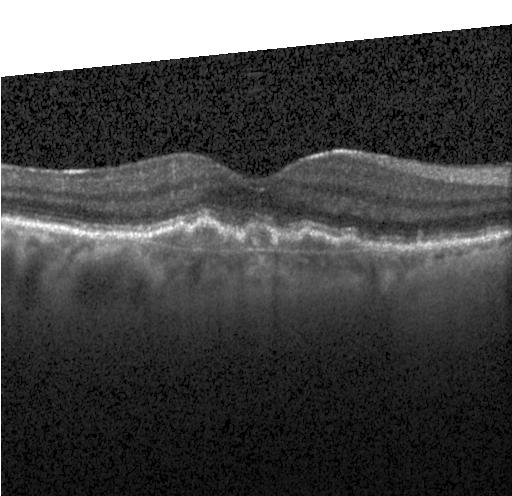 OCT scan showing CNV.